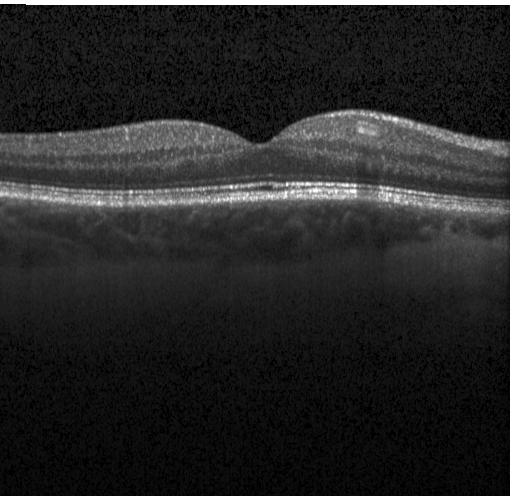 Retinal OCT B-scan, macular scan, spectral-domain optical coherence tomography, Heidelberg Spectralis — This B-scan demonstrates no evidence of CNV, DME, or drusen.